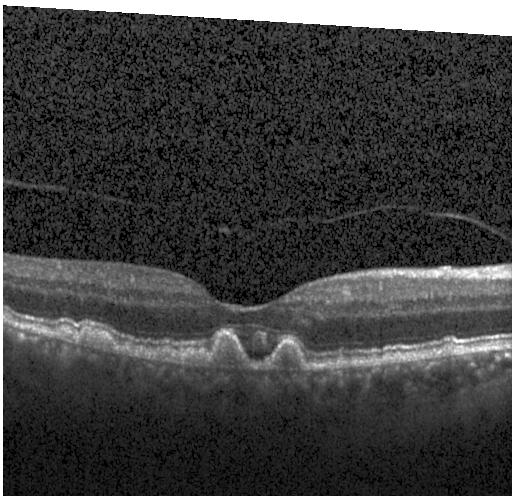
Spectral-domain OCT B-scan: a choroidal neovascular membrane.